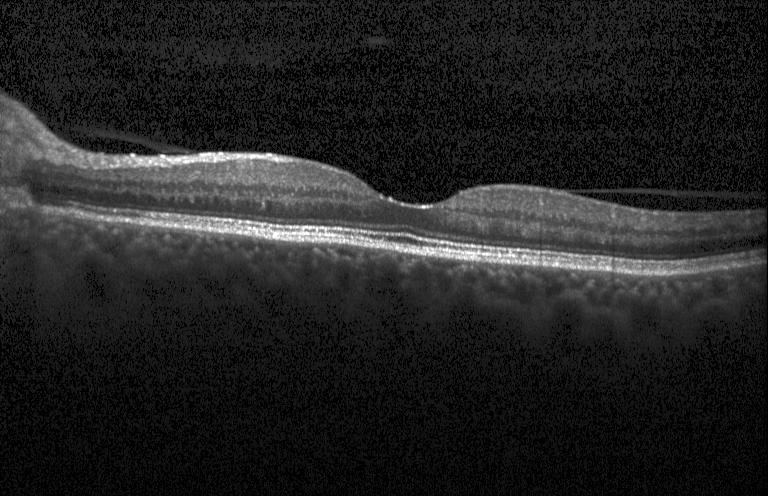

Retinal OCT B-scan.
OCT finding: no choroidal neovascularization, diabetic macular edema, or drusen.